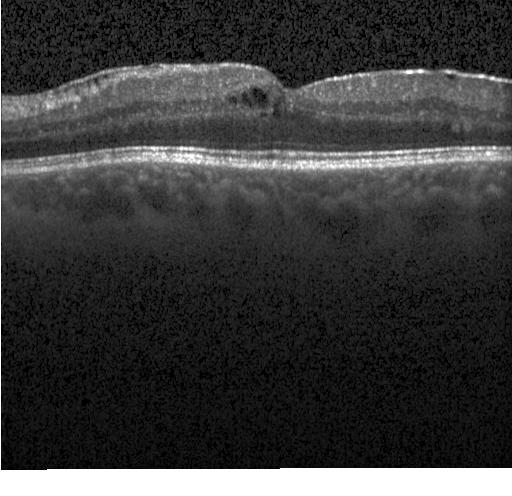 Heidelberg Spectralis OCT system. Optical coherence tomography B-scan. SD-OCT. Through the macula
Finding: diabetic macular edema (DME).